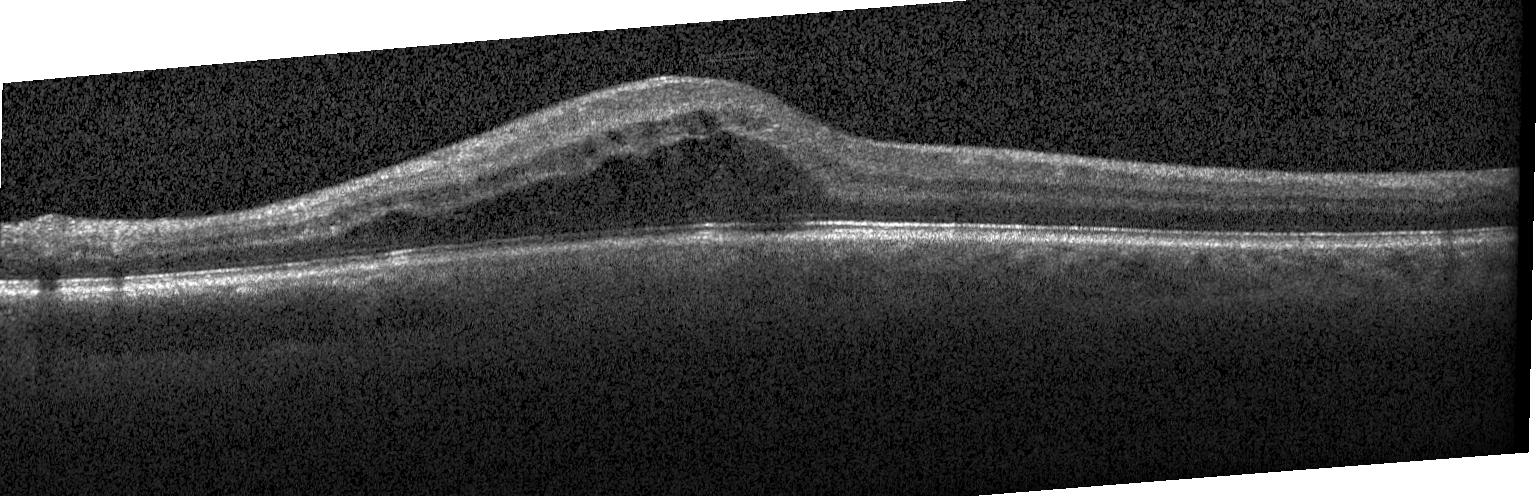 Retinal OCT cross-section, through the macula.
OCT finding: diabetic macular edema.